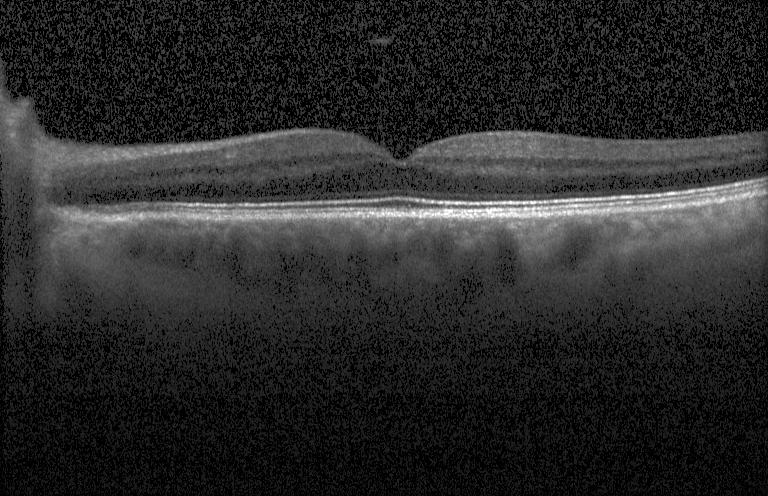 SD-OCT, horizontal scan through the fovea, acquired on a Heidelberg Spectralis, retinal OCT B-scan. No choroidal neovascularization, diabetic macular edema, or drusen.